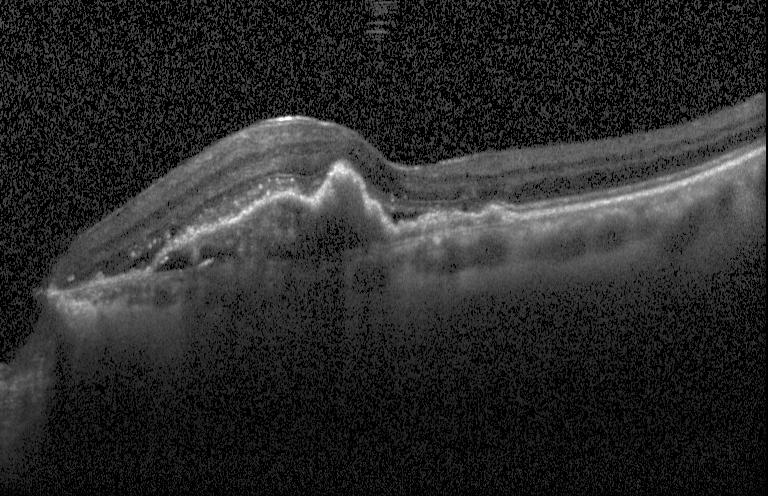 This B-scan demonstrates choroidal neovascularization (CNV).